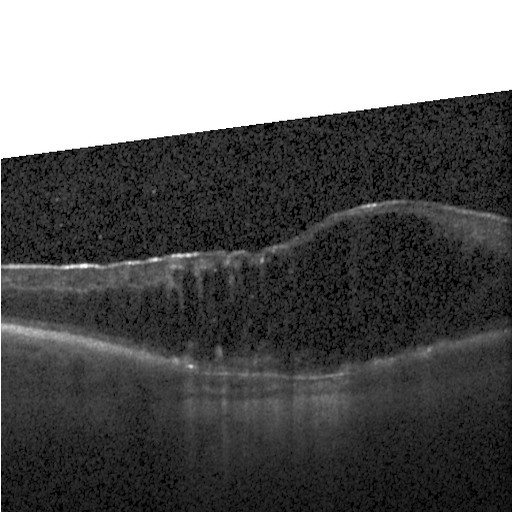 OCT line scan. Diagnosis: DME.